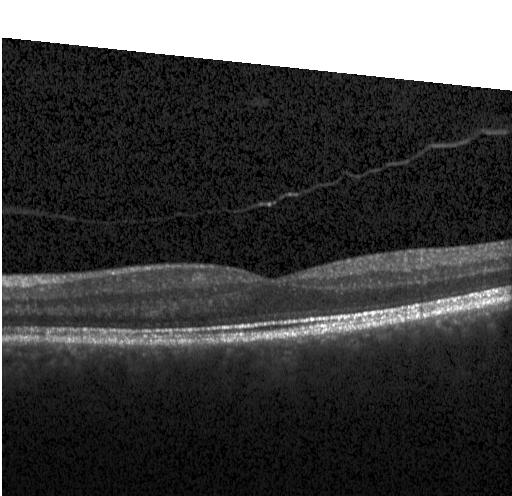
Optical coherence tomography B-scan · spectral-domain OCT. Macular OCT: no CNV, no DME, and no drusen.